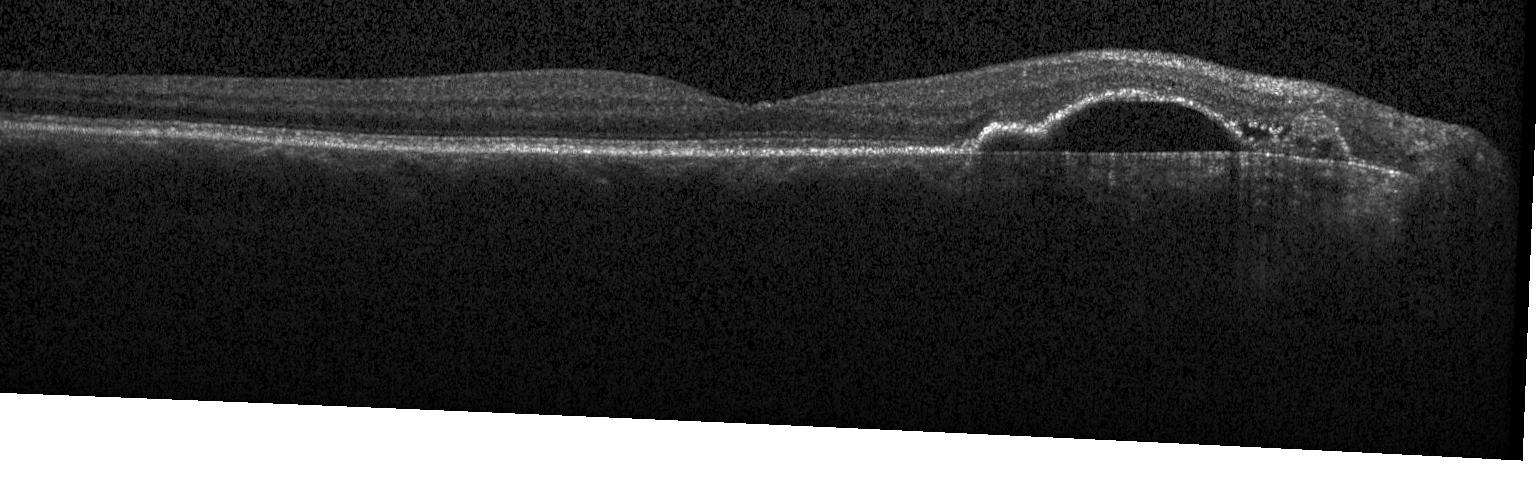
SD-OCT · optical coherence tomography scan · instrument: Heidelberg Spectralis · centered on the fovea
This B-scan demonstrates choroidal neovascularization.